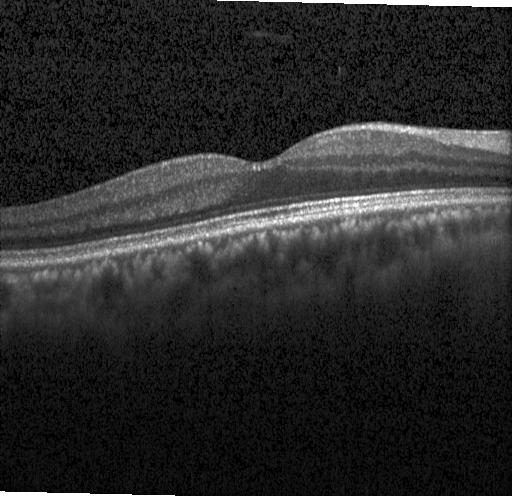

Retinal OCT B-scan.
This B-scan demonstrates neither CNV, DME, nor drusen.